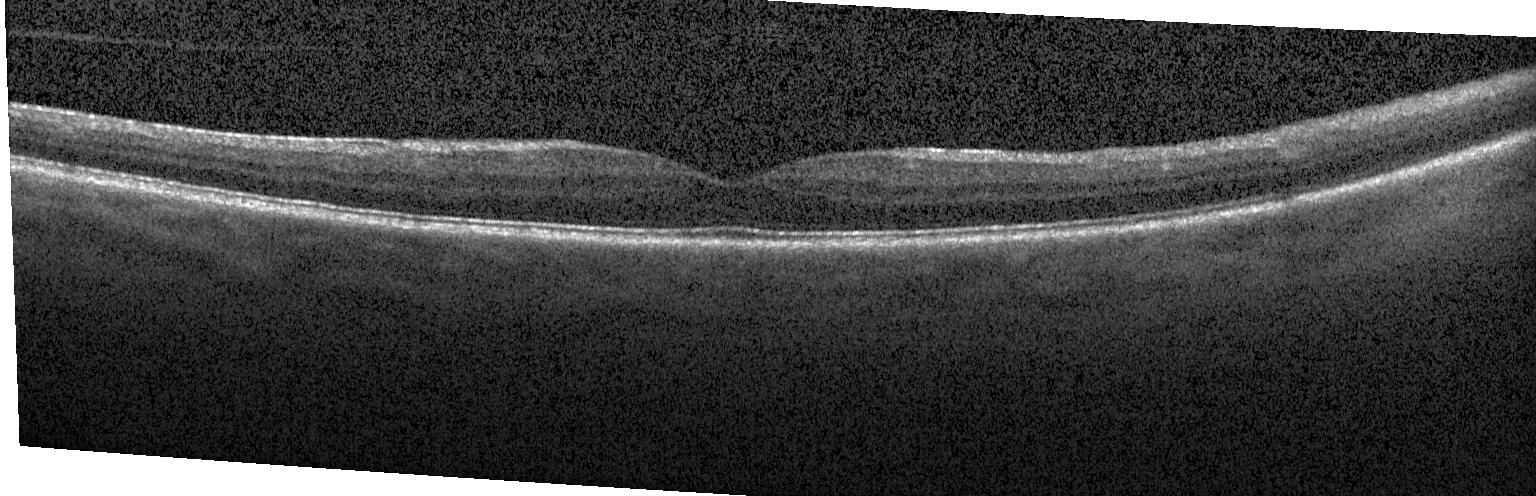

Retinal OCT B-scan · instrument: Heidelberg Spectralis — No evidence of CNV, DME, or drusen.